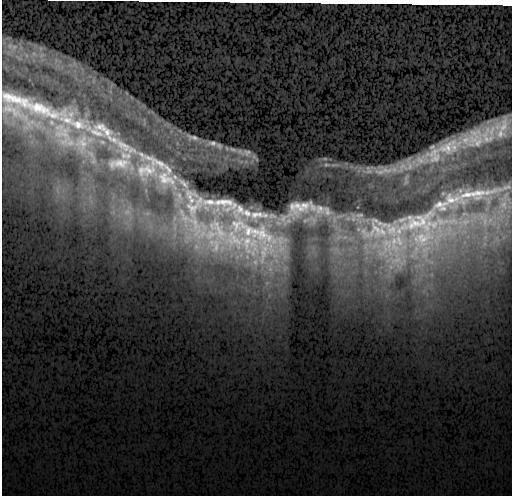

Optical coherence tomography B-scan, fovea-centered — This B-scan demonstrates a choroidal neovascular membrane.